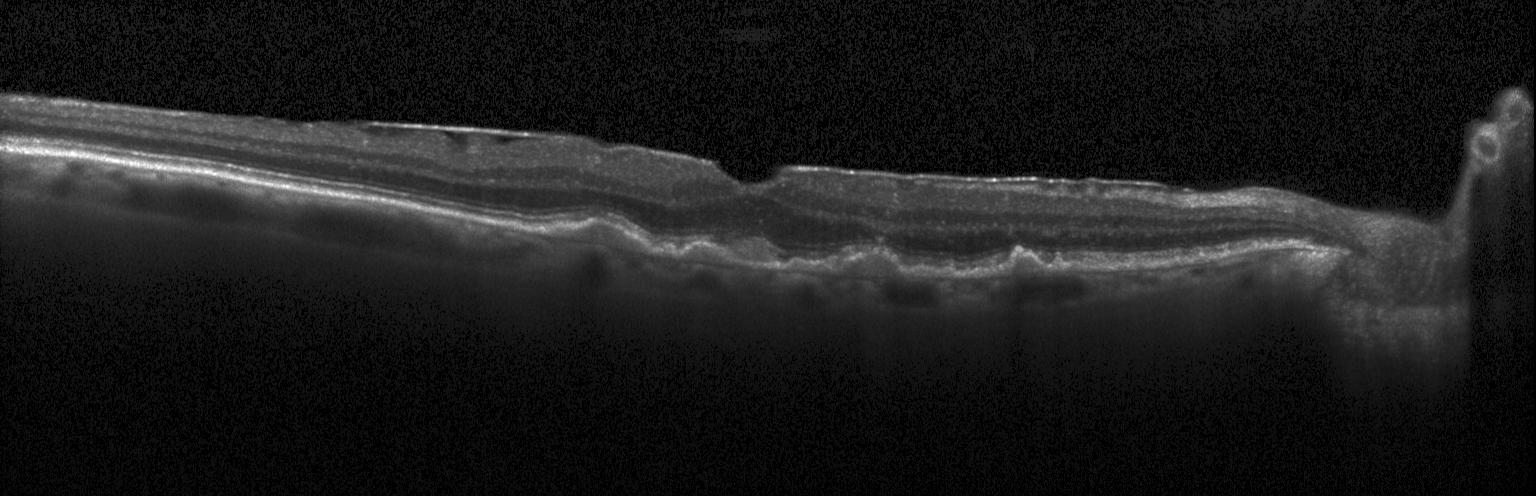
Optical coherence tomography scan · spectral-domain optical coherence tomography
Diagnosis: sub-RPE drusenoid deposits.